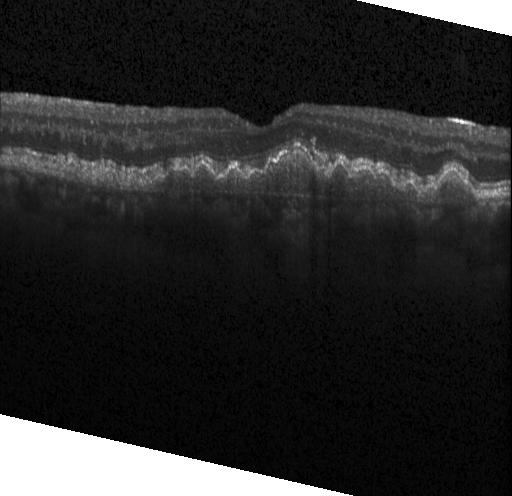
Optical coherence tomography B-scan. Acquired on a Heidelberg Spectralis. Assessment: choroidal neovascularization (CNV).